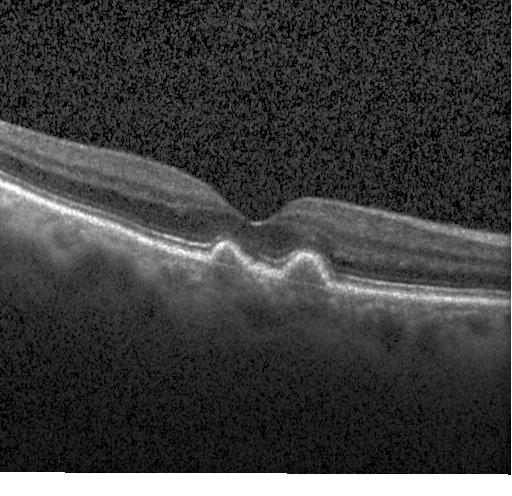 Diagnosis: drusen.